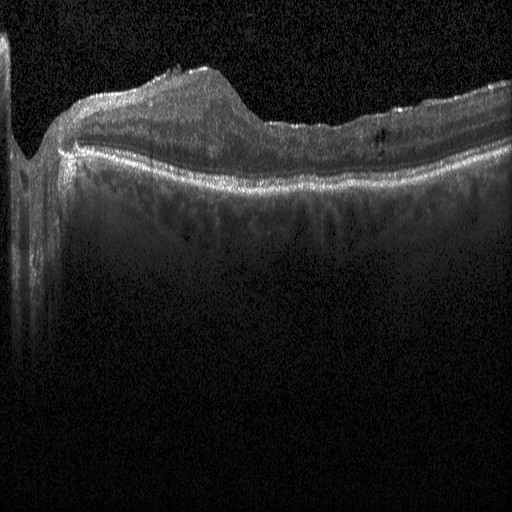
Instrument: Heidelberg Spectralis, spectral-domain optical coherence tomography, fovea-centered, OCT line scan.
Diabetic macular edema (DME).